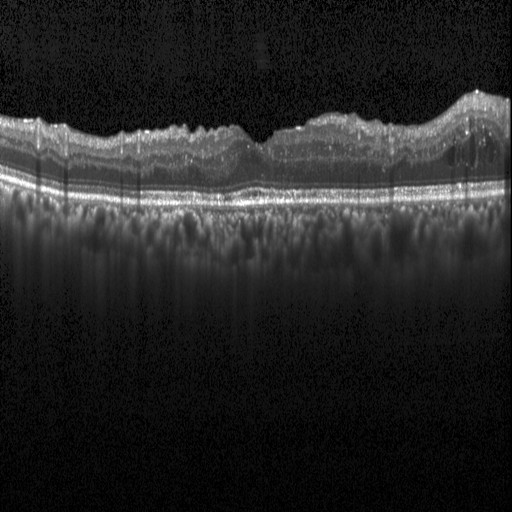

OCT line scan
Finding: DME.